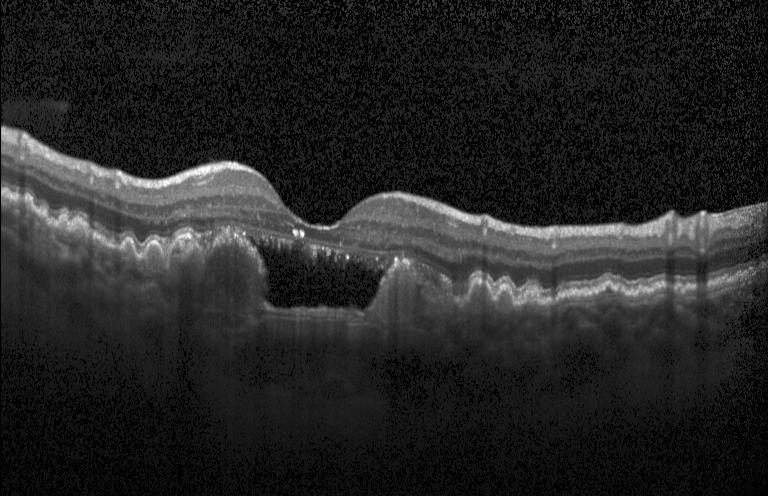 Retinal OCT B-scan. Spectral-domain OCT — Finding: choroidal neovascularization.